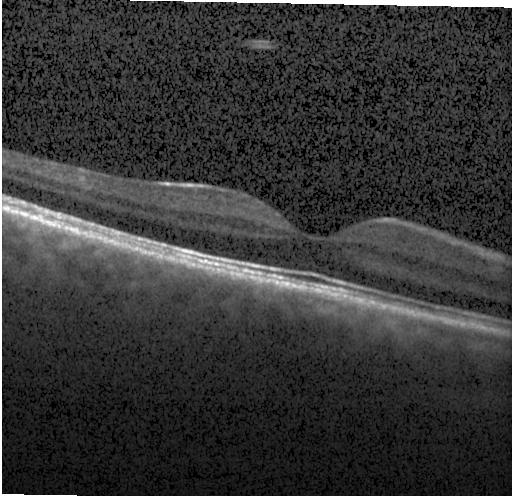
Heidelberg Spectralis OCT system. Retinal OCT cross-section. Spectral-domain OCT
This B-scan demonstrates no choroidal neovascularization, diabetic macular edema, or drusen.